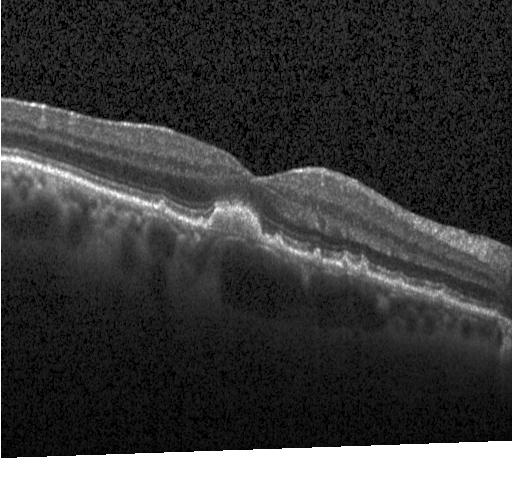

Dx: multiple drusen.